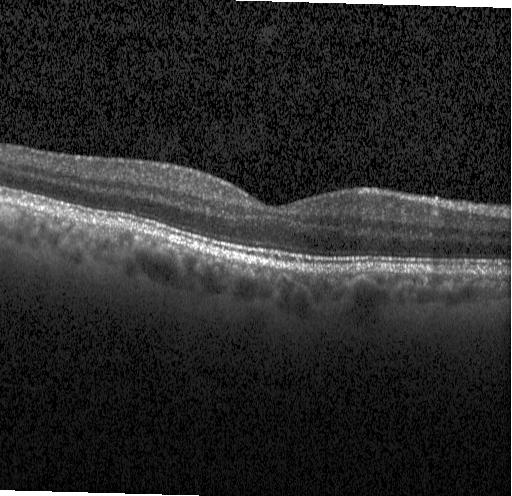
OCT line scan. Impression: no choroidal neovascularization, diabetic macular edema, or drusen.